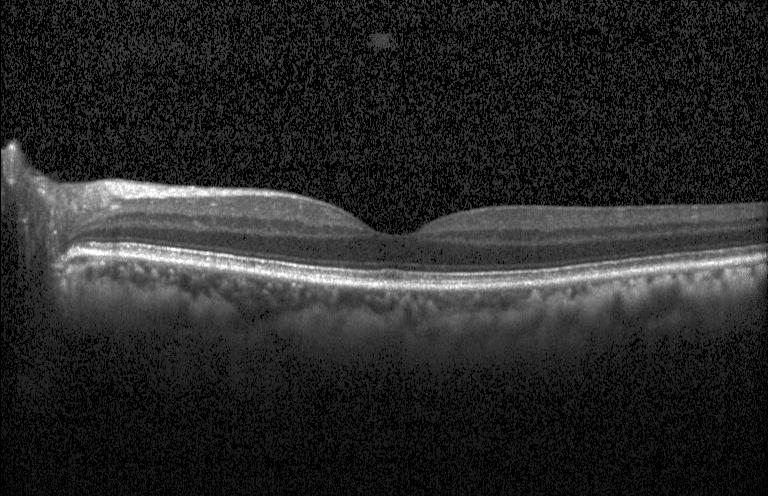 Optical coherence tomography scan; centered on the fovea; acquired on a Heidelberg Spectralis.
The scan shows no evidence of choroidal neovascularization, diabetic macular edema, or drusen.